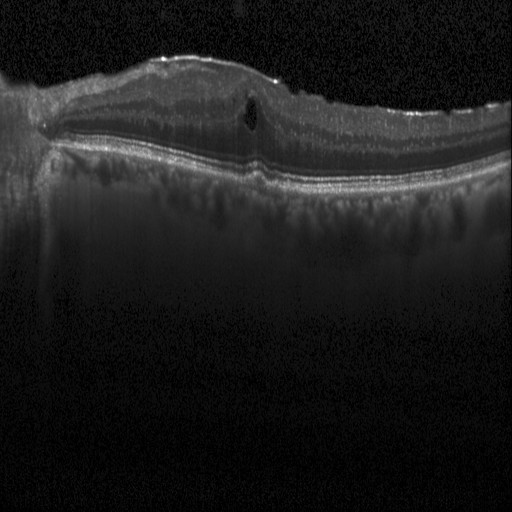 Instrument: Heidelberg Spectralis · OCT line scan · SD-OCT · through the macula. This B-scan demonstrates DME.